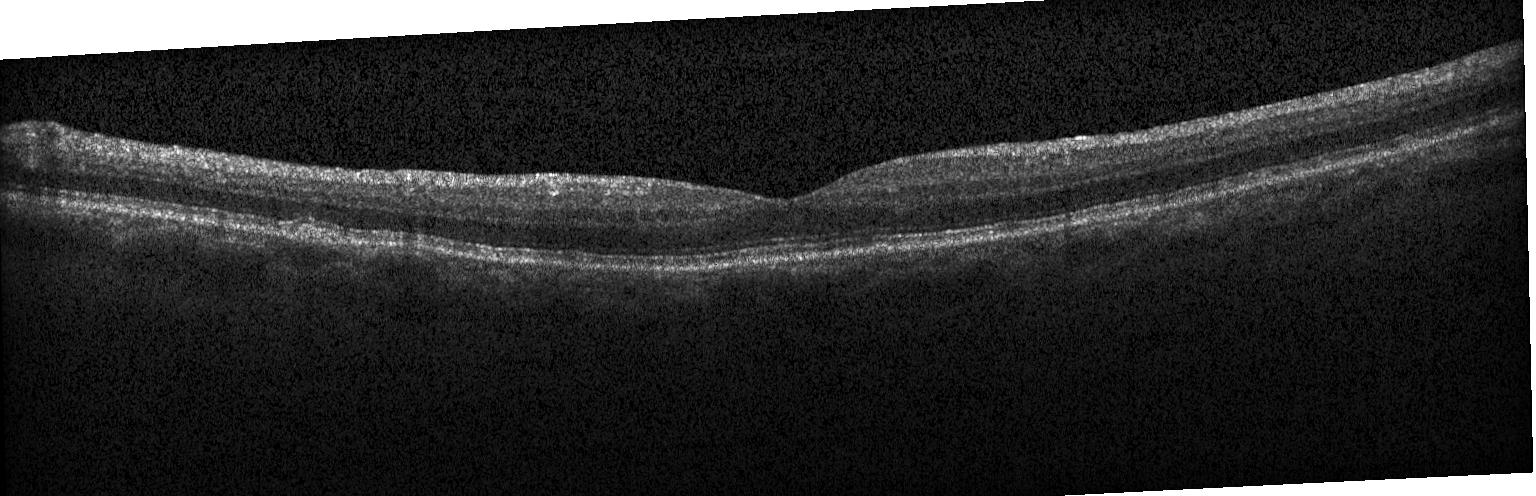

Finding: sub-RPE drusenoid deposits.